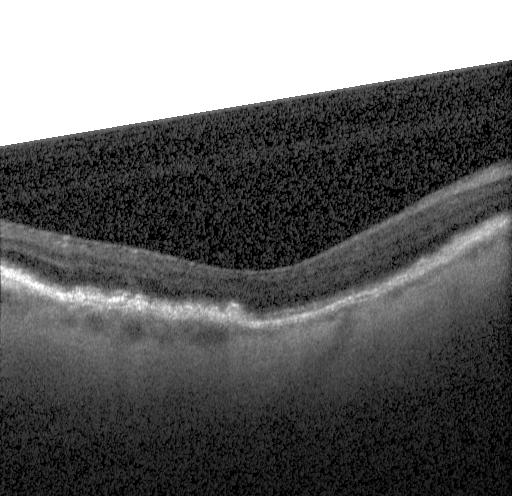
Retinal OCT B-scan
Diagnosis: CNV.